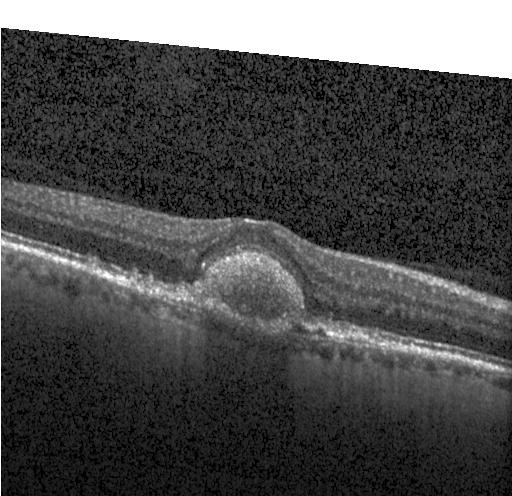 Fovea-centered. Acquired on a Heidelberg Spectralis. Spectral-domain optical coherence tomography. Retinal OCT cross-section
Assessment: a choroidal neovascular membrane.